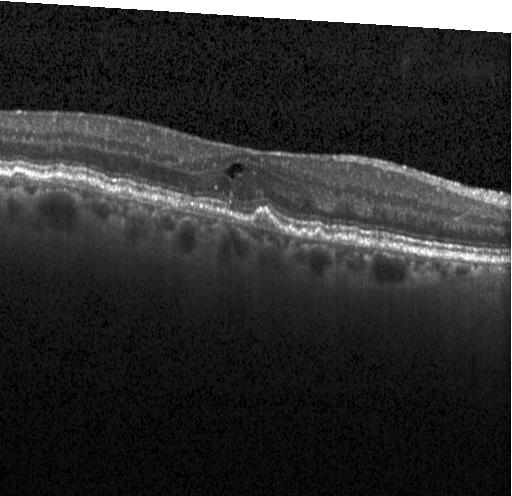 This B-scan demonstrates a choroidal neovascular membrane.